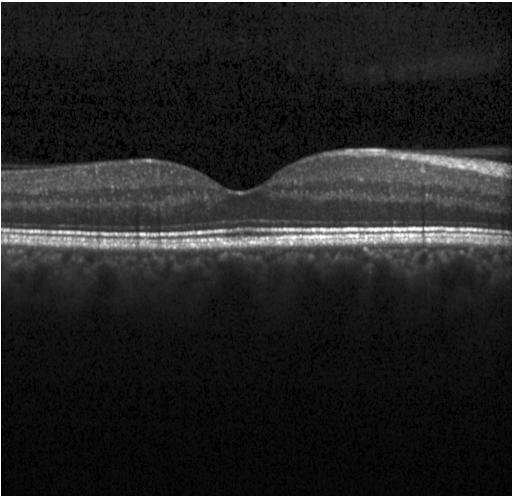
Centered on the fovea. SD-OCT. Retinal OCT B-scan. Heidelberg Spectralis — Impression: neither choroidal neovascularization, diabetic macular edema, nor drusen.